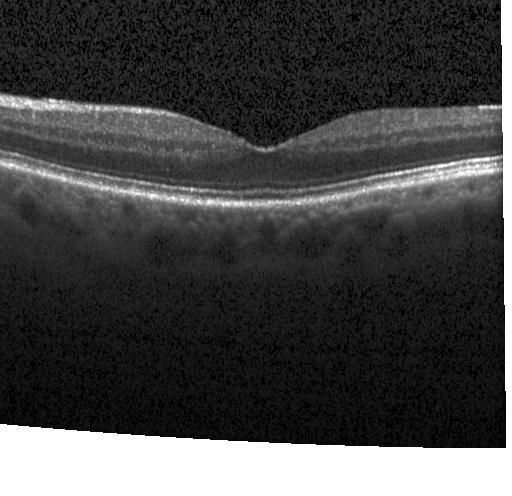

Retinal OCT B-scan; Heidelberg Spectralis; SD-OCT; fovea-centered
Finding: neither CNV, DME, nor drusen.